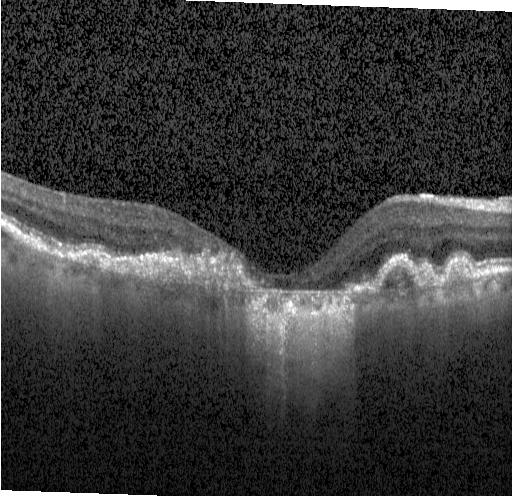
Diagnosis: a choroidal neovascular membrane.